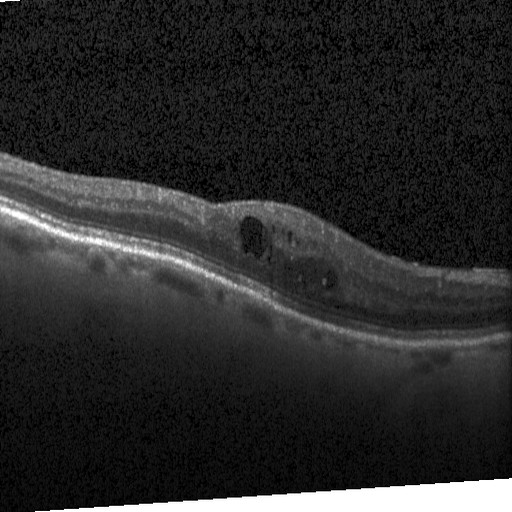
Diagnosis: DME.